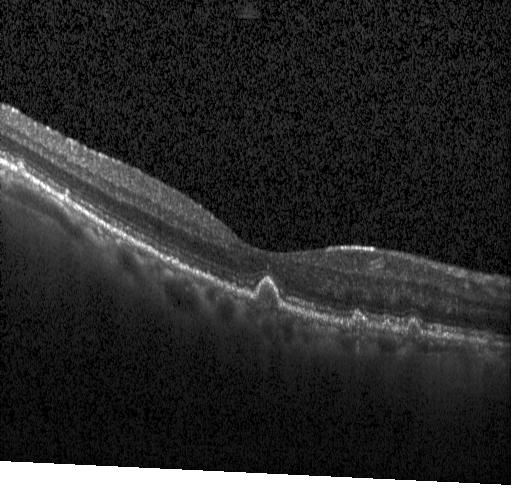 Acquired on a Heidelberg Spectralis; horizontal scan through the fovea; SD-OCT; OCT line scan — This B-scan demonstrates multiple drusen.